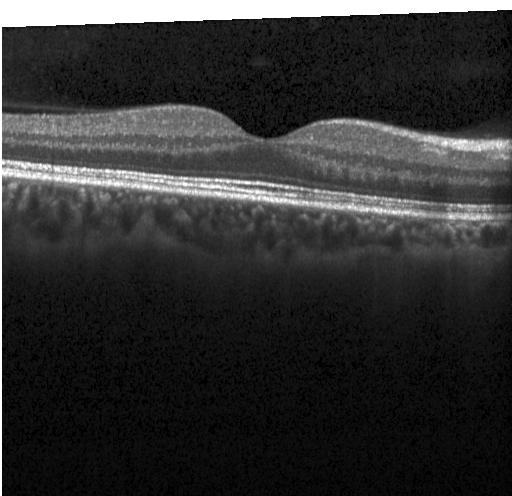
Optical coherence tomography B-scan; fovea-centered; acquired on a Heidelberg Spectralis
Diagnosis: no choroidal neovascularization, diabetic macular edema, or drusen.